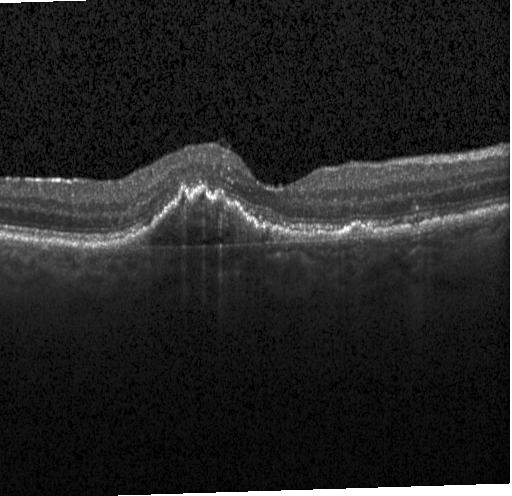
Heidelberg Spectralis; spectral-domain OCT; retinal OCT cross-section. Assessment: a choroidal neovascular membrane.